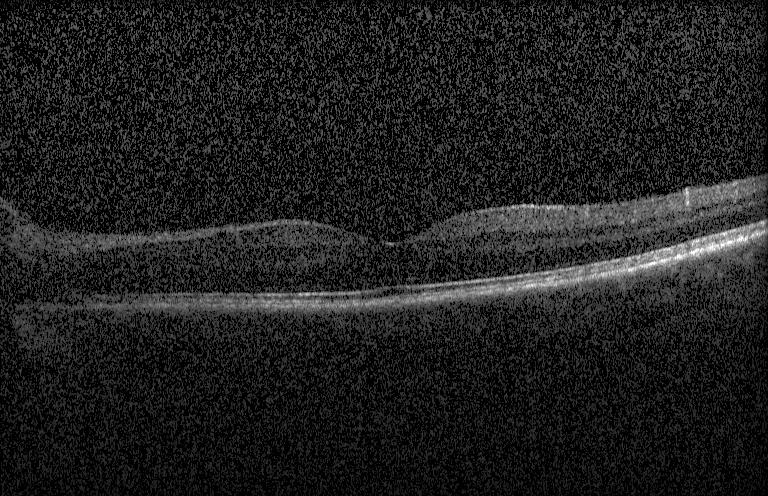

OCT line scan; spectral-domain OCT; horizontal scan through the fovea
Finding: neither choroidal neovascularization, diabetic macular edema, nor drusen.